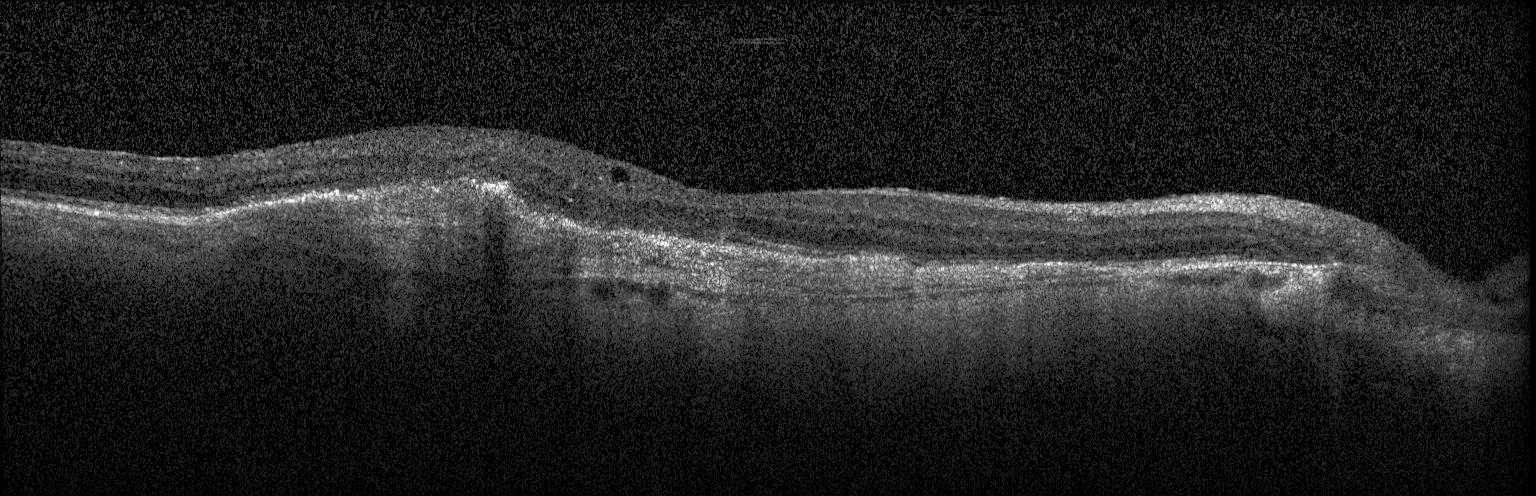 Fovea-centered · retinal OCT cross-section · Heidelberg Spectralis.
Finding: choroidal neovascularization (CNV).